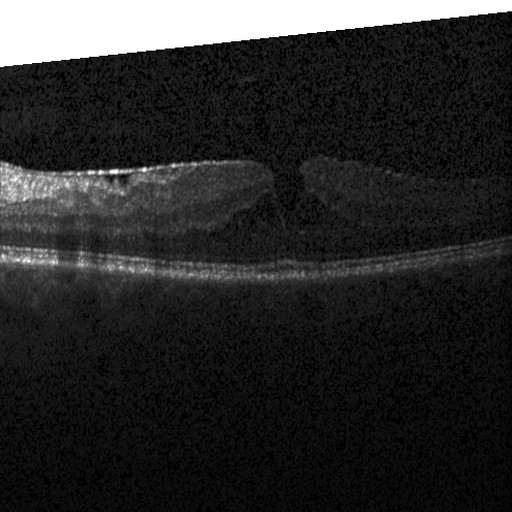

OCT B-scan. Heidelberg Spectralis OCT system. Assessment: diabetic macular edema (DME).